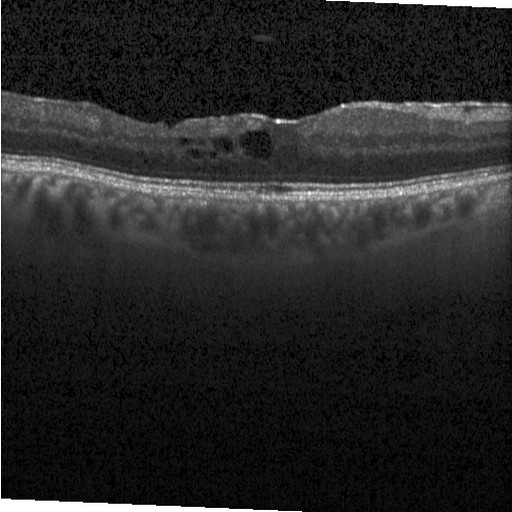 Retinal OCT cross-section; through the macula.
Diabetic macular edema (DME).